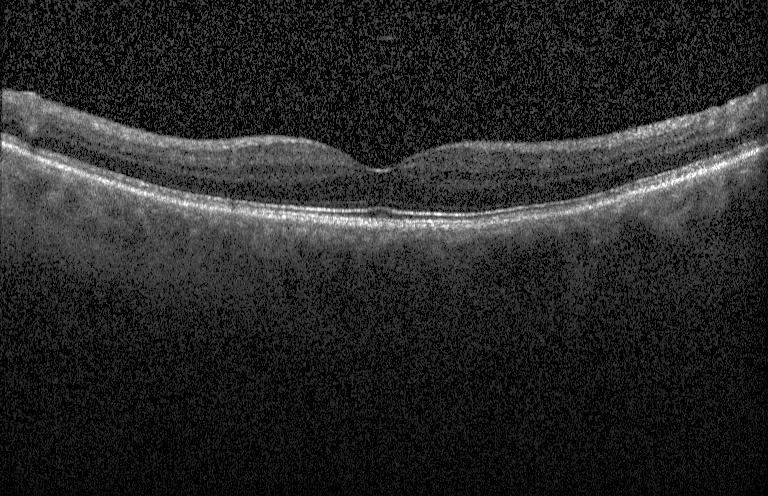
Heidelberg Spectralis · centered on the fovea · optical coherence tomography scan · SD-OCT — No CNV, no DME, and no drusen.